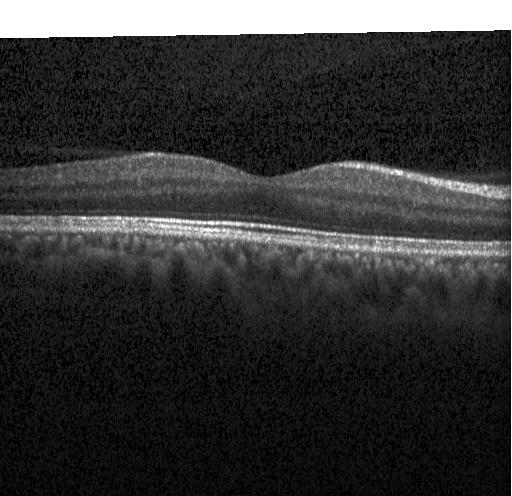

Macular scan. Heidelberg Spectralis OCT system. Retinal OCT B-scan
Macular OCT: no evidence of choroidal neovascularization, diabetic macular edema, or drusen.